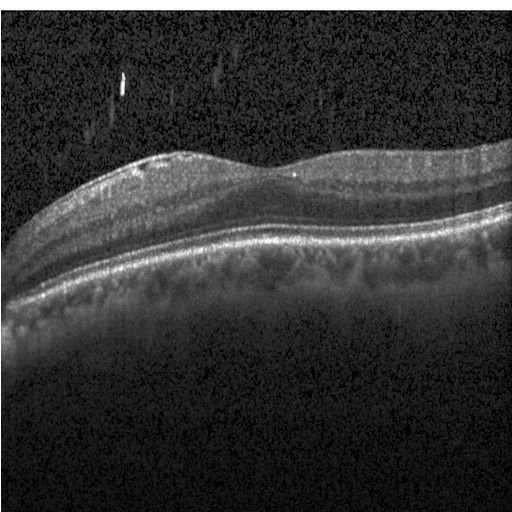
Spectral-domain OCT B-scan: DME.